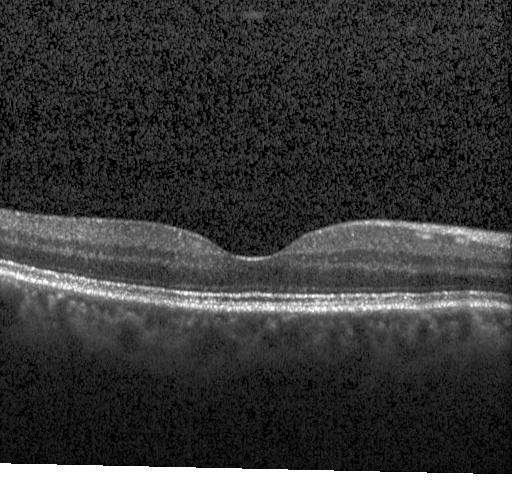
OCT line scan. SD-OCT. Macular scan — Assessment: no evidence of choroidal neovascularization, diabetic macular edema, or drusen.